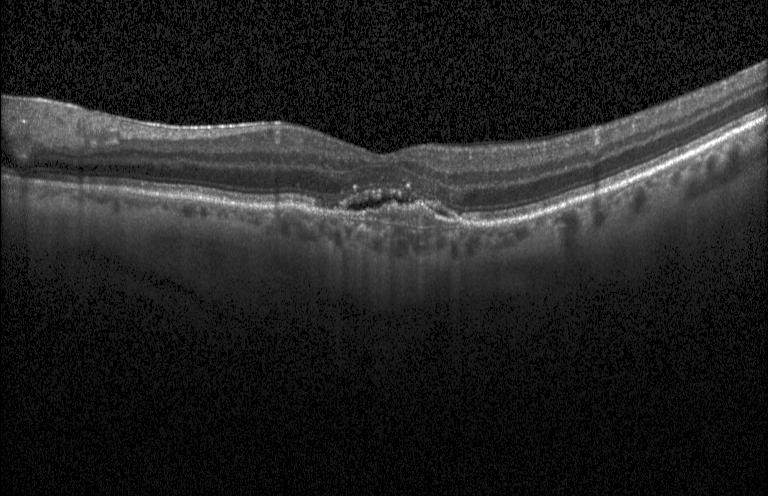 Horizontal scan through the fovea; retinal OCT B-scan
Macular OCT: a choroidal neovascular membrane.